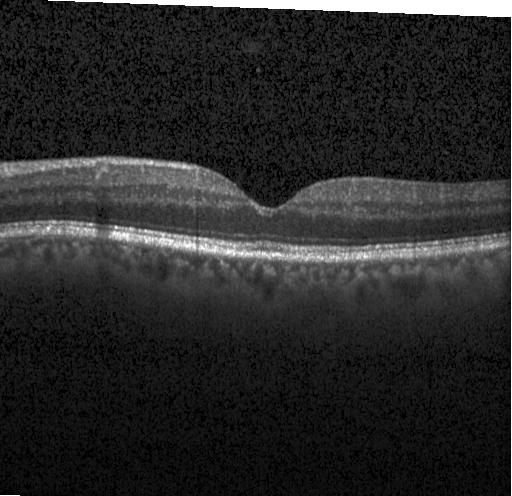

Spectral-domain OCT. Centered on the fovea. Optical coherence tomography B-scan. Instrument: Heidelberg Spectralis
Finding: no choroidal neovascularization, diabetic macular edema, or drusen.